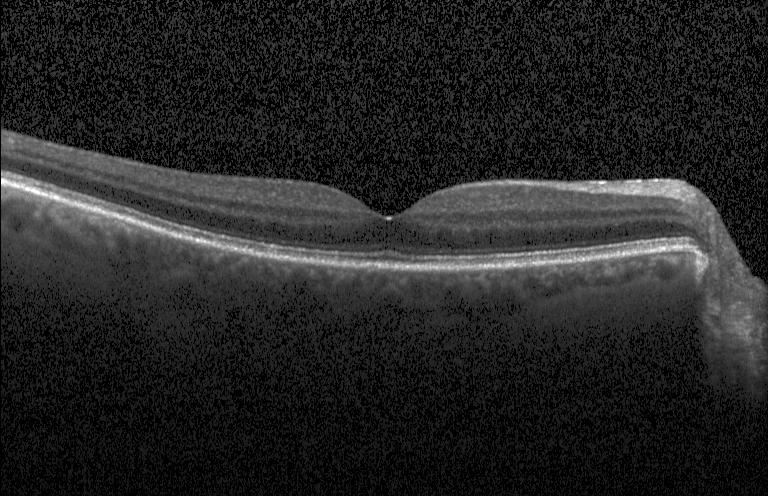
This B-scan demonstrates no choroidal neovascularization, diabetic macular edema, or drusen.